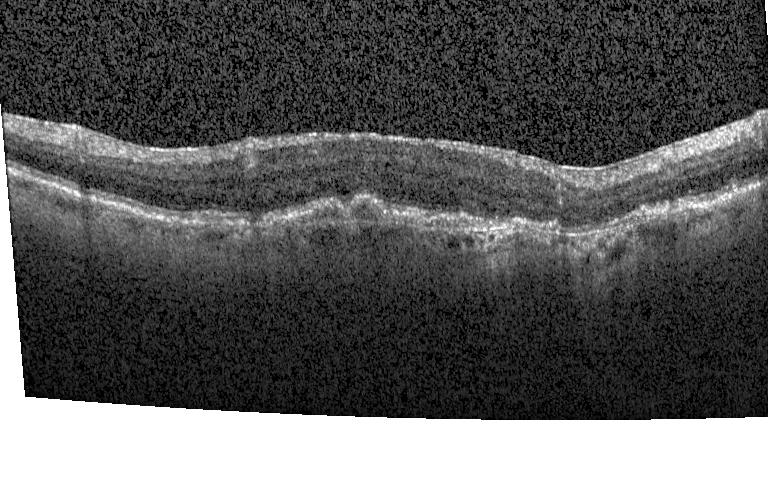 Centered on the fovea; Heidelberg Spectralis OCT system; OCT B-scan; spectral-domain OCT
Macular OCT: a choroidal neovascular membrane.